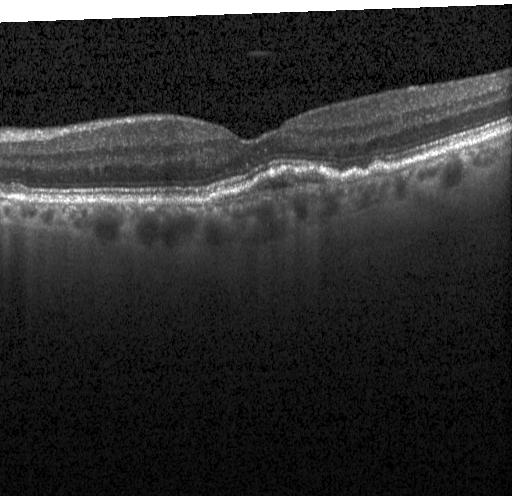 Horizontal scan through the fovea, Heidelberg Spectralis, optical coherence tomography B-scan, SD-OCT
Assessment: choroidal neovascularization (CNV).